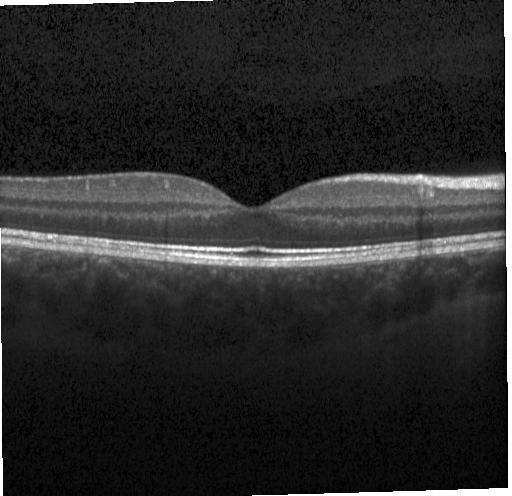

Assessment: neither CNV, DME, nor drusen.